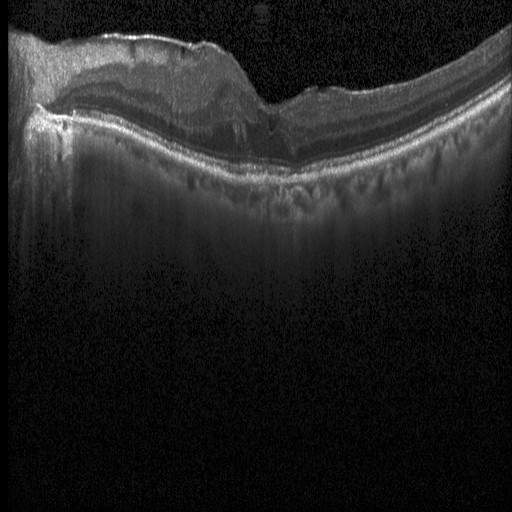 Retinal OCT cross-section, Heidelberg Spectralis, macular scan, SD-OCT
Macular OCT: diabetic macular edema.